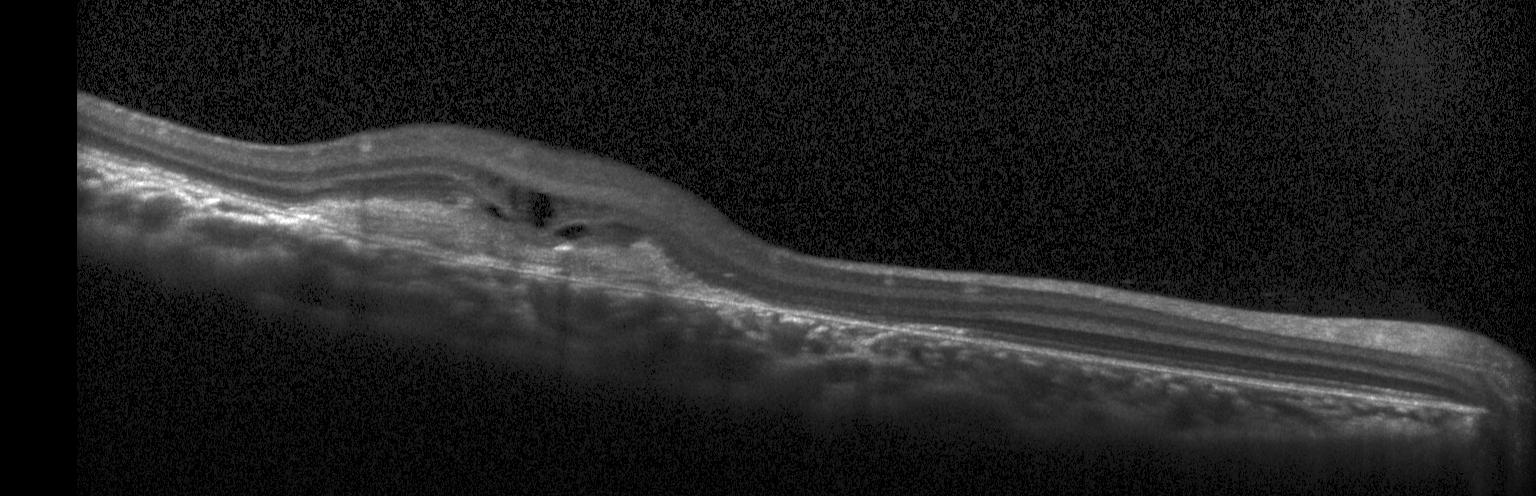

Assessment: choroidal neovascularization.